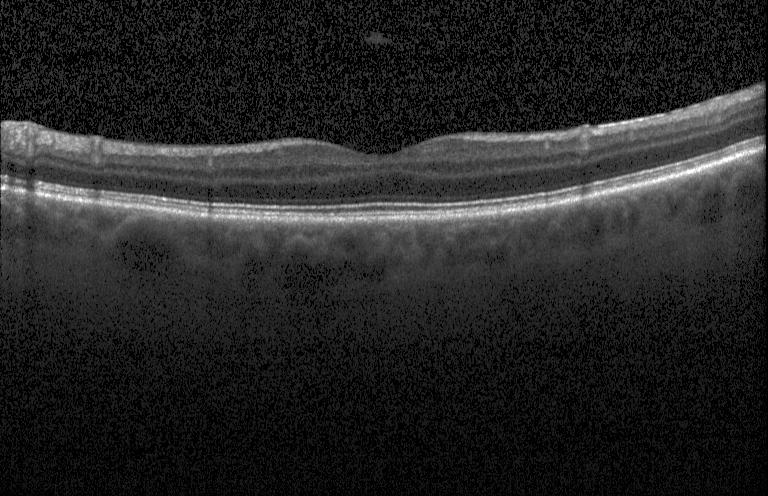 Retinal OCT cross-section showing no choroidal neovascularization, diabetic macular edema, or drusen.